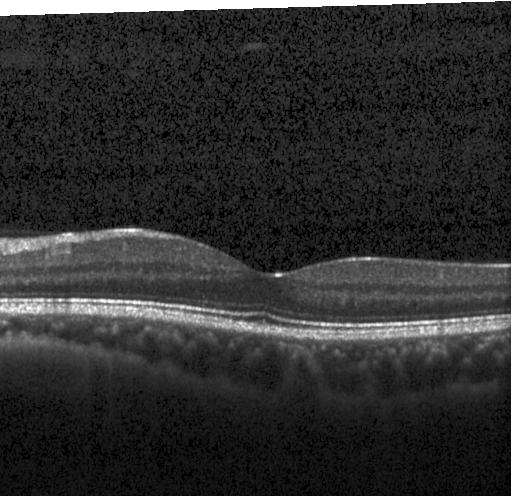
Fovea-centered. Optical coherence tomography B-scan.
Finding: neither choroidal neovascularization, diabetic macular edema, nor drusen.